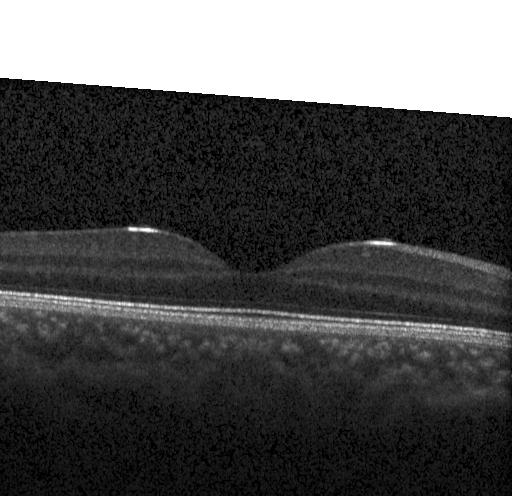

Heidelberg Spectralis OCT system. Spectral-domain OCT. Macular scan. Optical coherence tomography scan. Impression: no choroidal neovascularization, diabetic macular edema, or drusen.